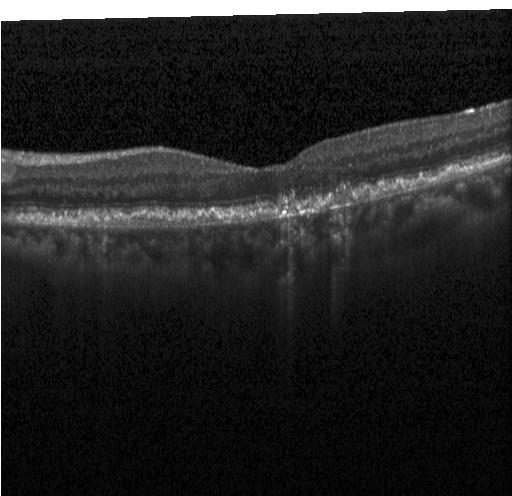 Spectral-domain OCT, optical coherence tomography B-scan, macular scan.
This B-scan demonstrates multiple drusen.